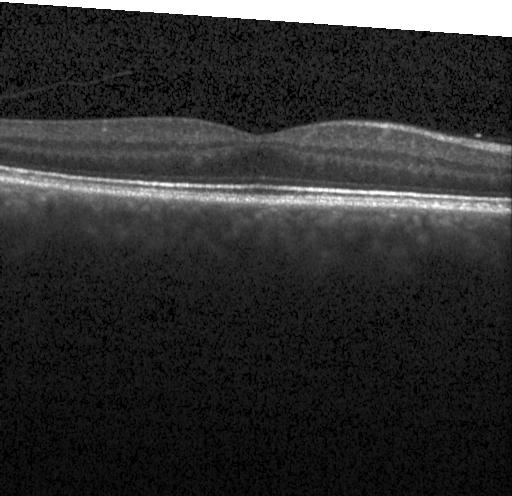 Spectral-domain OCT B-scan: no evidence of choroidal neovascularization, diabetic macular edema, or drusen.